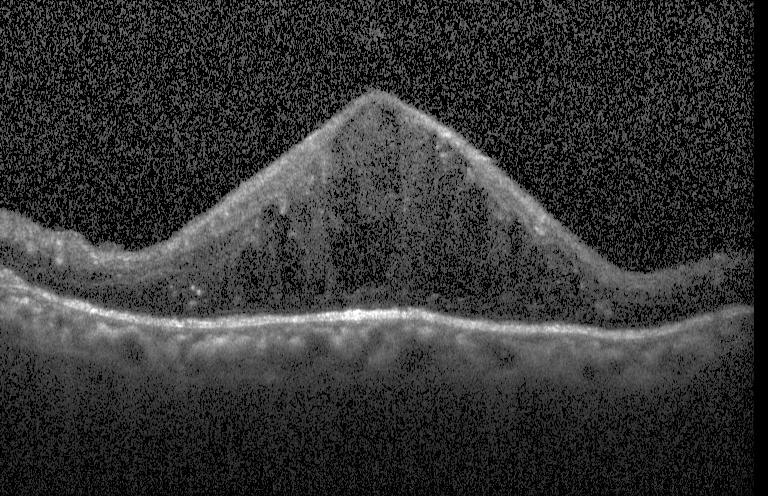

Diagnosis: DME.